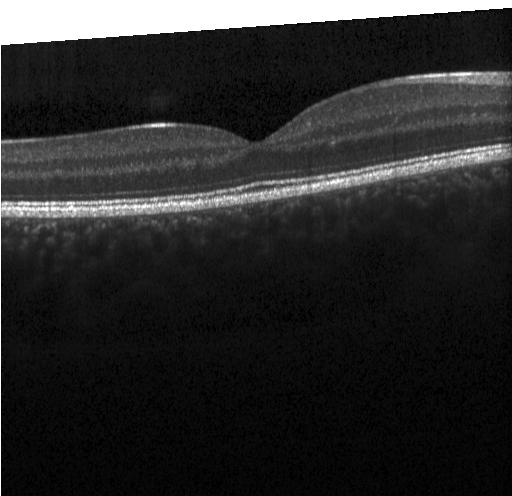 Instrument: Heidelberg Spectralis, optical coherence tomography B-scan, SD-OCT, macular scan.
Assessment: neither choroidal neovascularization, diabetic macular edema, nor drusen.